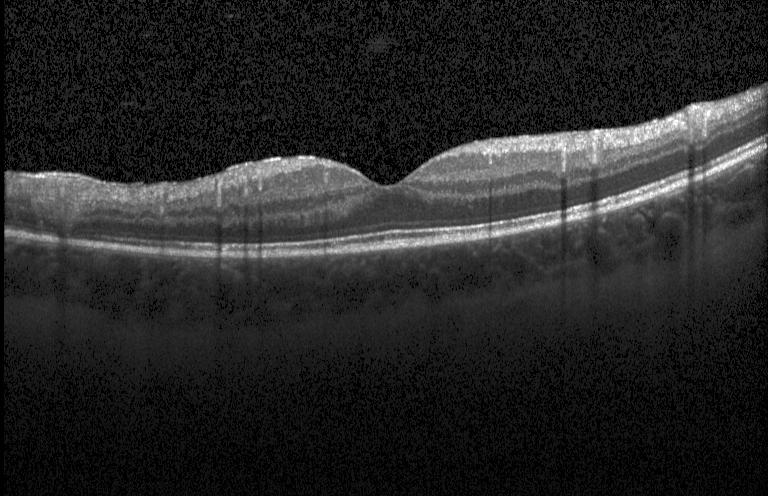

Macular OCT: no evidence of choroidal neovascularization, diabetic macular edema, or drusen.